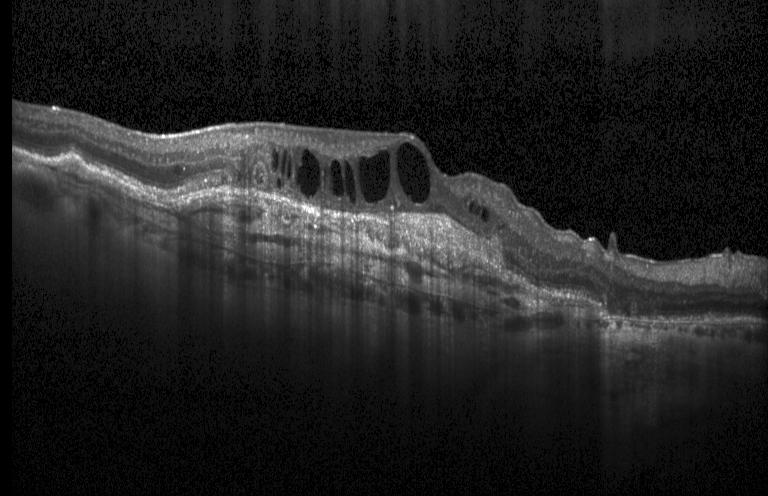
Diagnosis: a choroidal neovascular membrane.